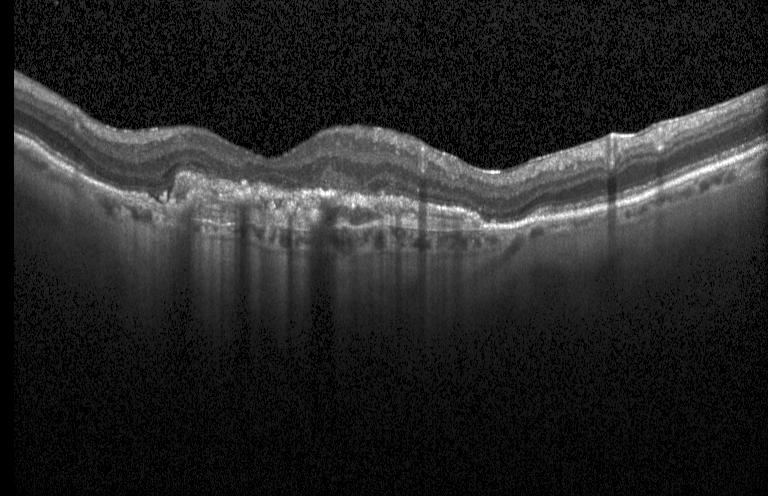

Heidelberg Spectralis OCT system. Retinal OCT cross-section. Through the macula. Spectral-domain optical coherence tomography. Assessment: choroidal neovascularization.